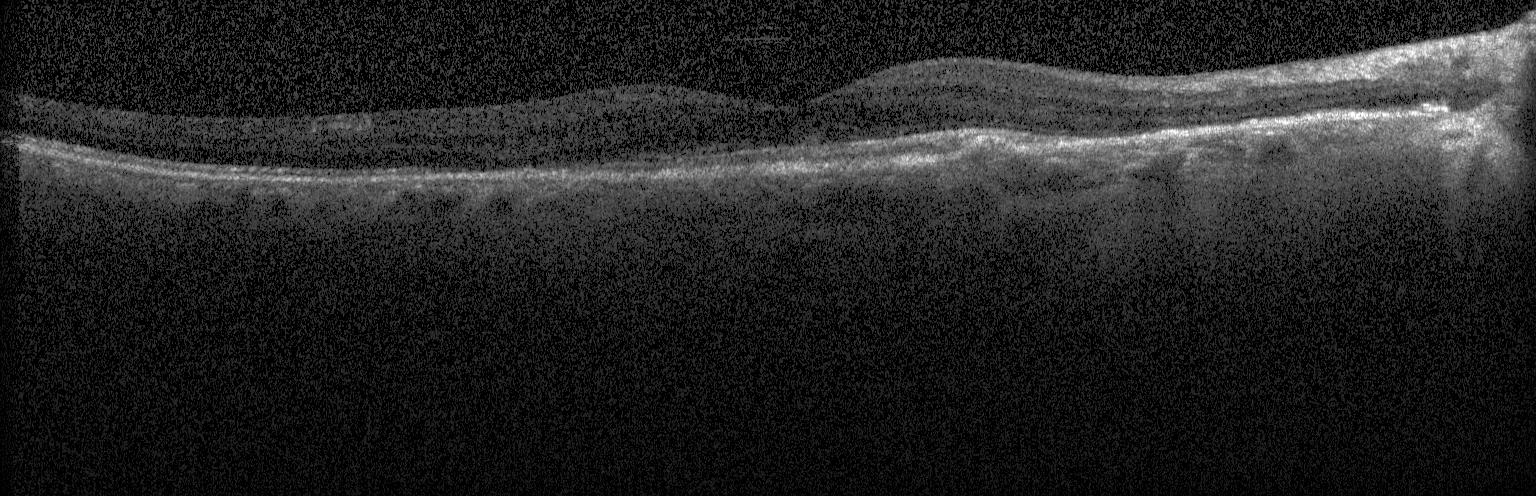

Retinal OCT cross-section showing a choroidal neovascular membrane.